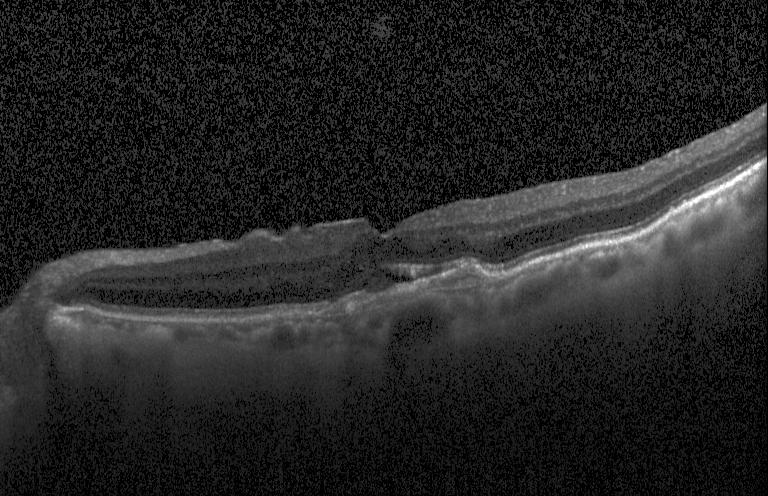
Diagnosis: choroidal neovascularization.